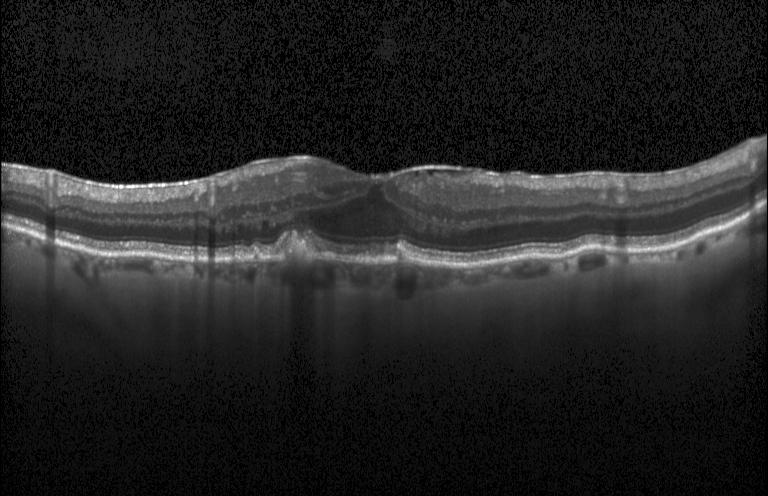
Optical coherence tomography B-scan — This B-scan demonstrates CNV.